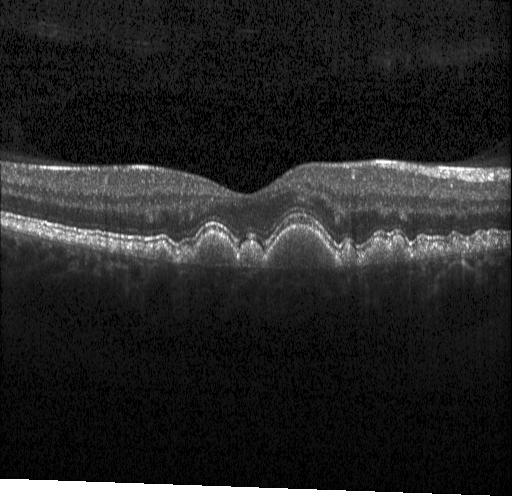

Spectral-domain OCT · OCT line scan · instrument: Heidelberg Spectralis · macular scan. Impression: drusen.